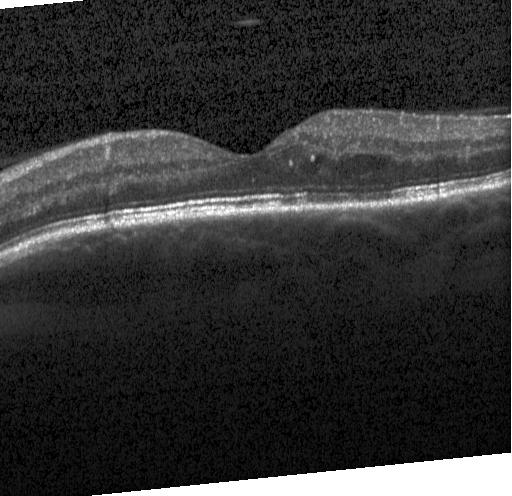

Retinal OCT B-scan, Heidelberg Spectralis, through the macula, spectral-domain optical coherence tomography — OCT finding: diabetic macular edema.